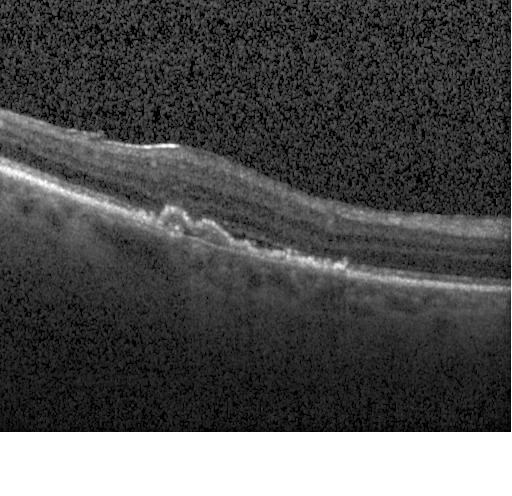 Finding: a choroidal neovascular membrane.